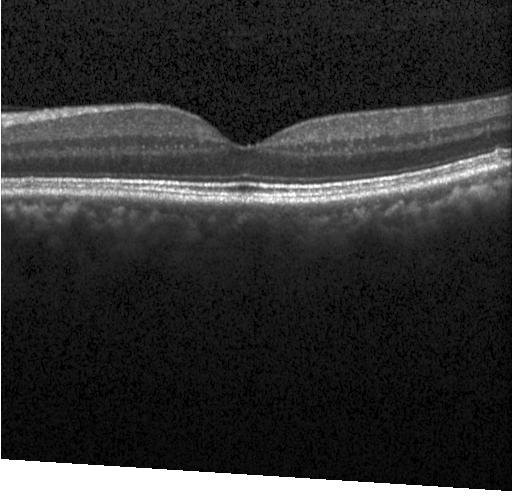 Retinal OCT B-scan — Assessment: neither choroidal neovascularization, diabetic macular edema, nor drusen.